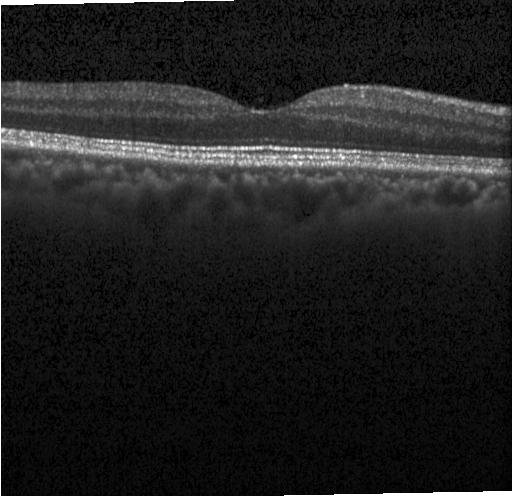
Heidelberg Spectralis · retinal OCT cross-section
The scan shows no evidence of choroidal neovascularization, diabetic macular edema, or drusen.